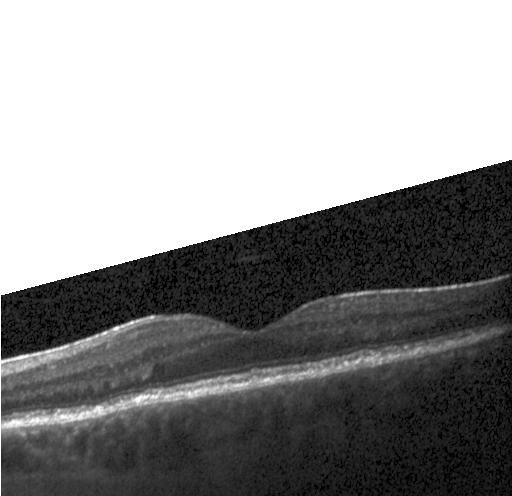

OCT B-scan. Macular scan. Diagnosis: neither choroidal neovascularization, diabetic macular edema, nor drusen.